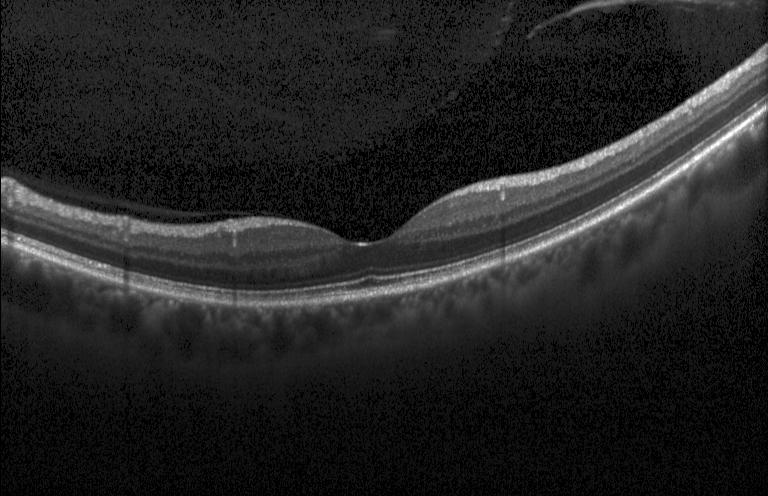

Retinal OCT cross-section. Assessment: no evidence of choroidal neovascularization, diabetic macular edema, or drusen.